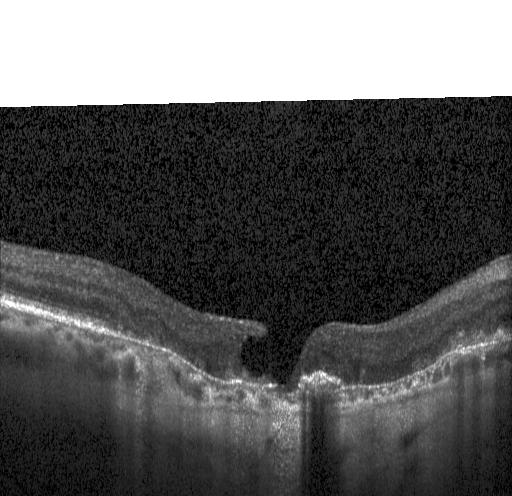
Macular OCT: choroidal neovascularization.